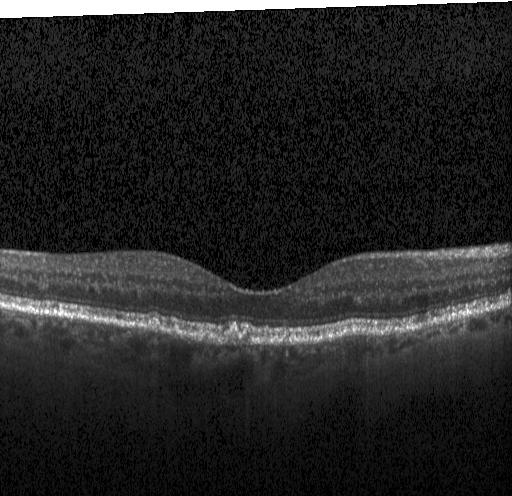

Assessment: sub-RPE drusenoid deposits.